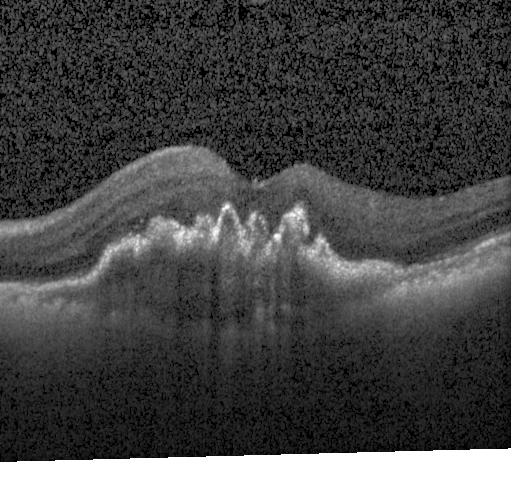

Retinal OCT B-scan; SD-OCT; centered on the fovea — Finding: a choroidal neovascular membrane.